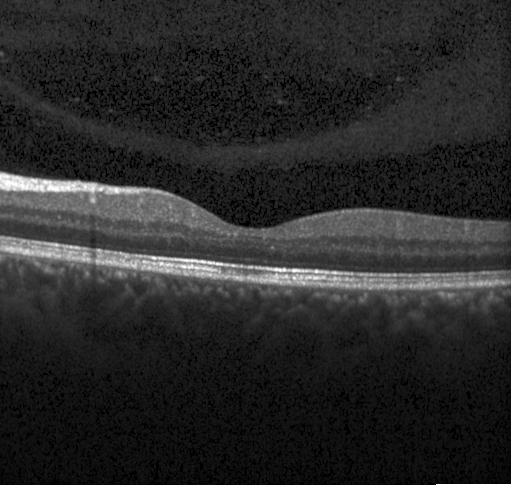 Diagnosis: neither choroidal neovascularization, diabetic macular edema, nor drusen.